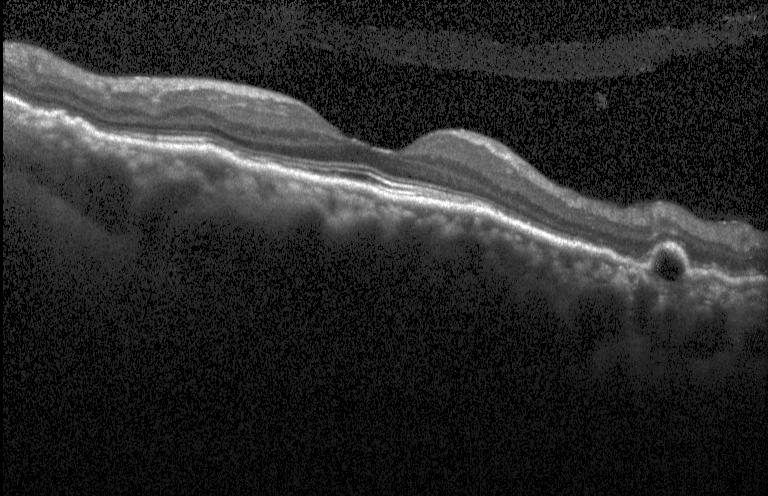
Macular OCT demonstrating choroidal neovascularization.